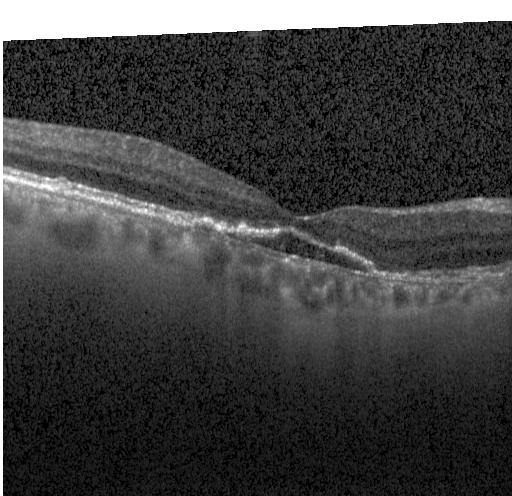

Spectral-domain optical coherence tomography · retinal OCT cross-section · through the macula · instrument: Heidelberg Spectralis.
Choroidal neovascularization (CNV).